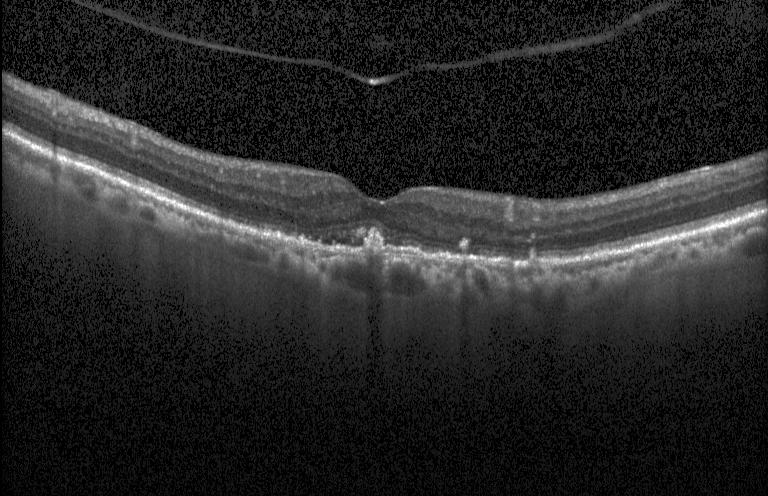
Spectral-domain optical coherence tomography · Heidelberg Spectralis · horizontal scan through the fovea · optical coherence tomography scan — Dx: choroidal neovascularization (CNV).